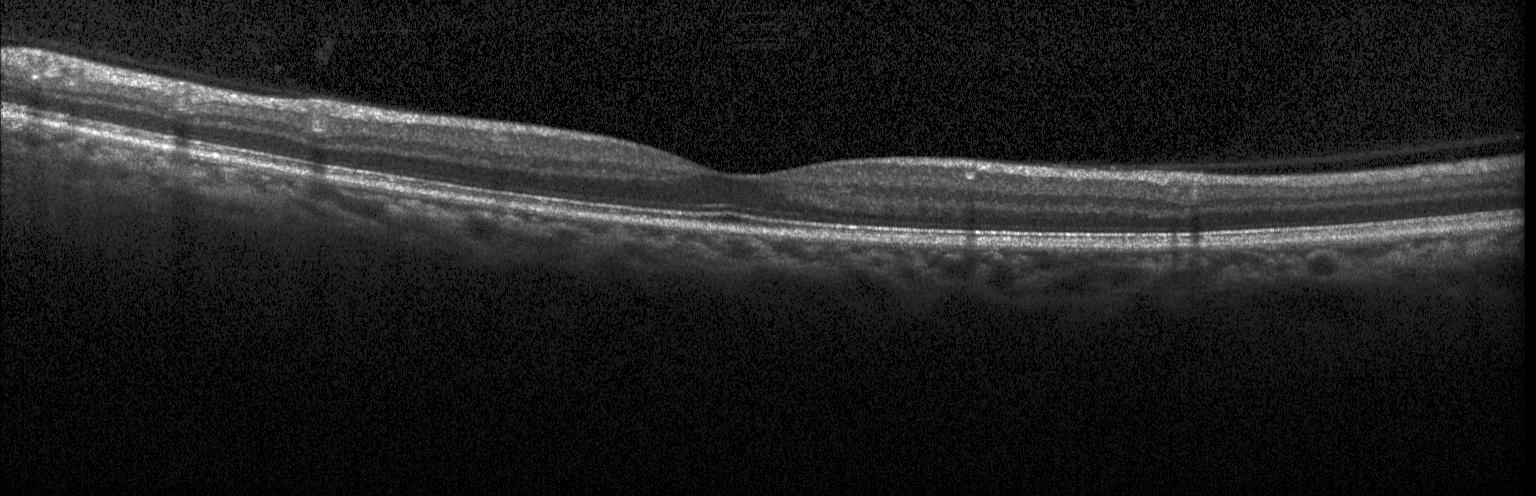
Assessment: no choroidal neovascularization, no diabetic macular edema, and no drusen.